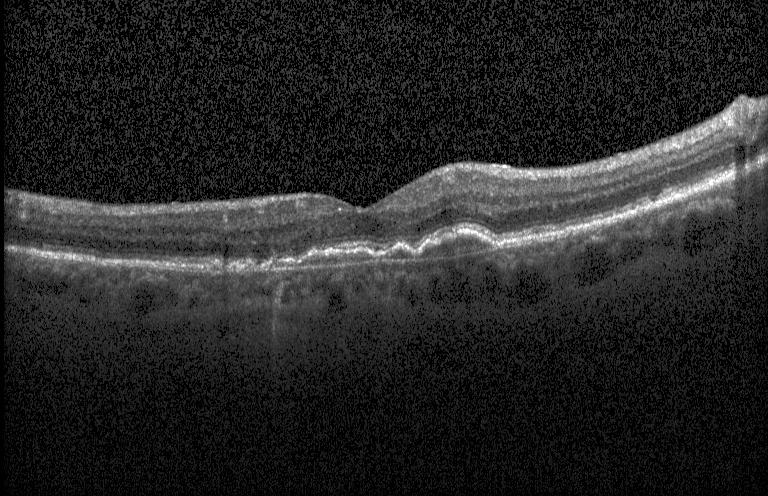

Spectral-domain OCT. Centered on the fovea. Retinal OCT cross-section
Diagnosis: choroidal neovascularization (CNV).